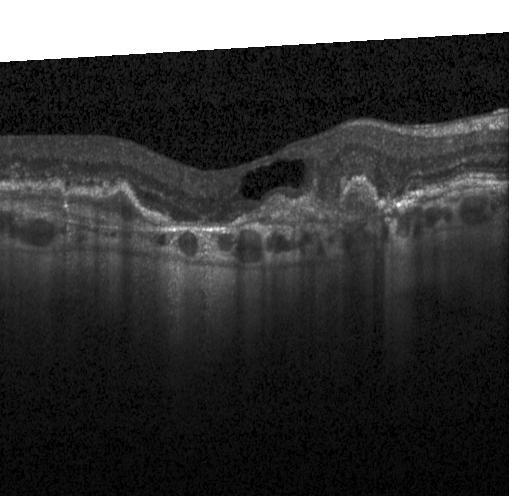

Heidelberg Spectralis OCT system. Spectral-domain OCT. Optical coherence tomography B-scan.
Finding: a choroidal neovascular membrane.